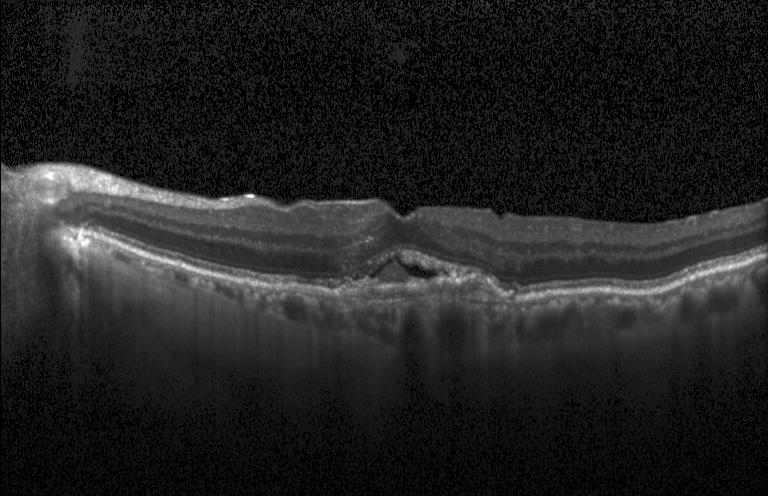
OCT scan showing choroidal neovascularization.